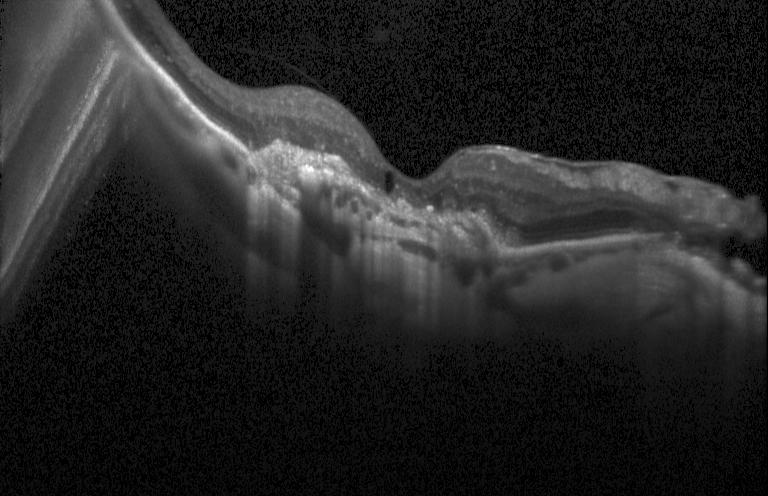 Diagnosis: choroidal neovascularization.